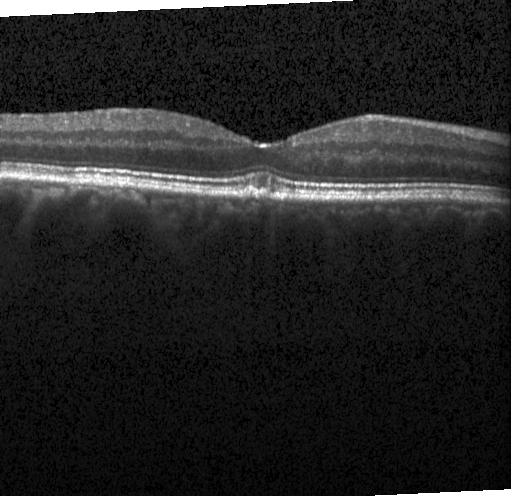
OCT line scan
The scan shows drusen.